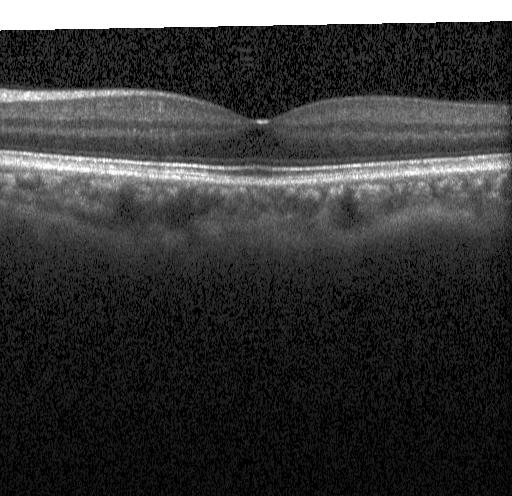
Heidelberg Spectralis. SD-OCT. Through the macula. Retinal OCT cross-section
Impression: neither choroidal neovascularization, diabetic macular edema, nor drusen.